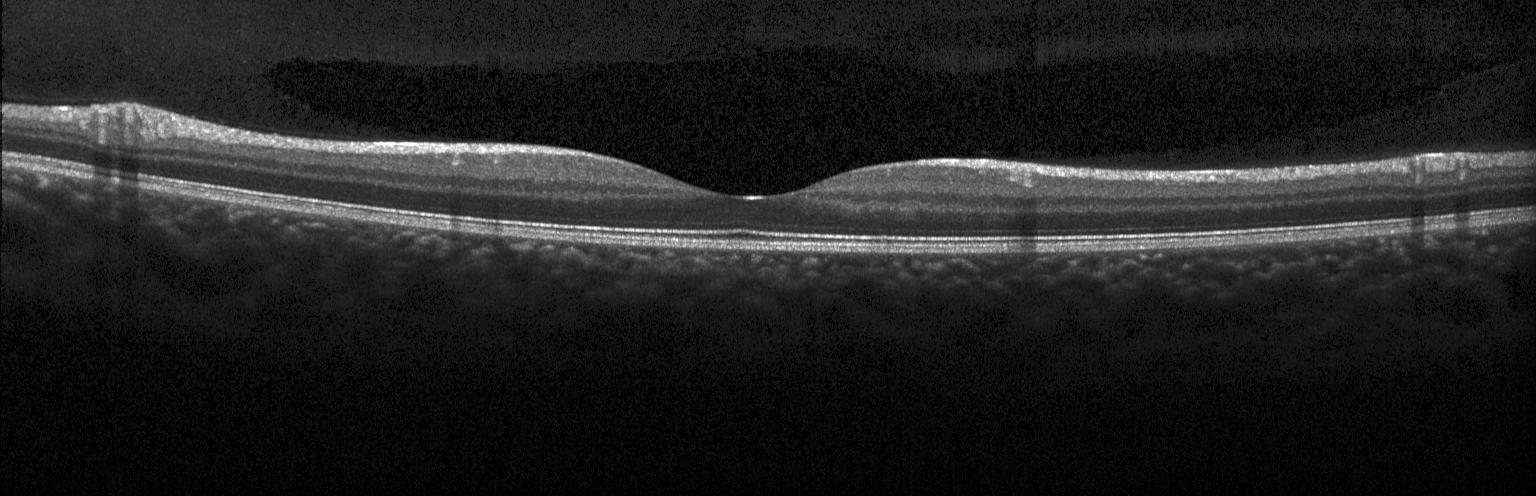 Spectral-domain OCT B-scan: no choroidal neovascularization, diabetic macular edema, or drusen.